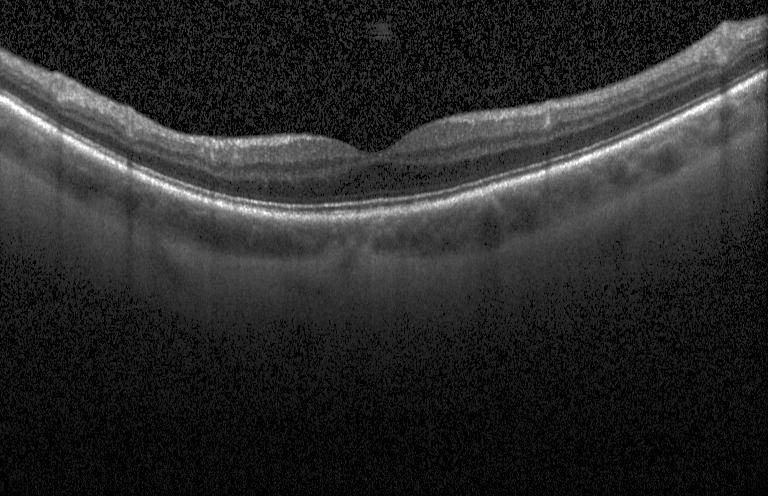
Optical coherence tomography scan, through the macula. Impression: no choroidal neovascularization, no diabetic macular edema, and no drusen.